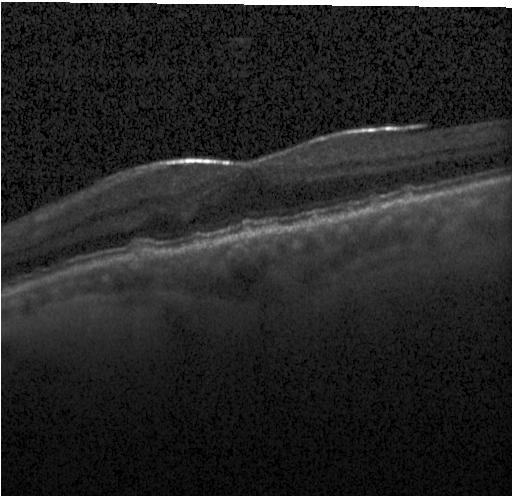

Heidelberg Spectralis OCT system, optical coherence tomography B-scan
Impression: drusen.